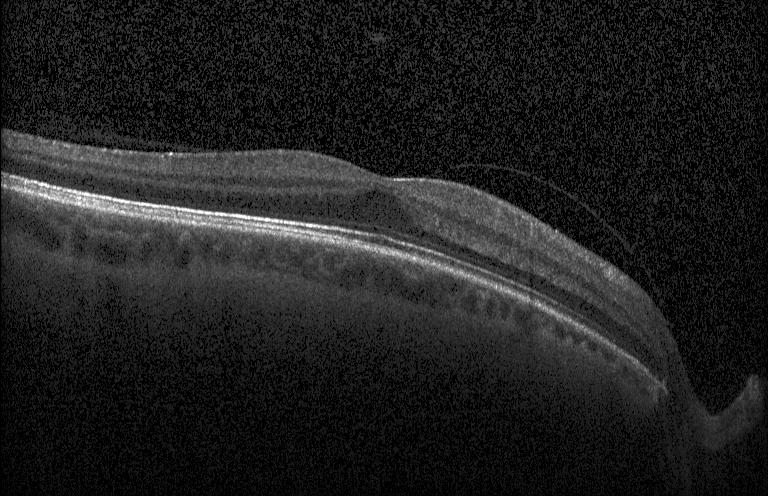
Retinal OCT cross-section showing no choroidal neovascularization, diabetic macular edema, or drusen.